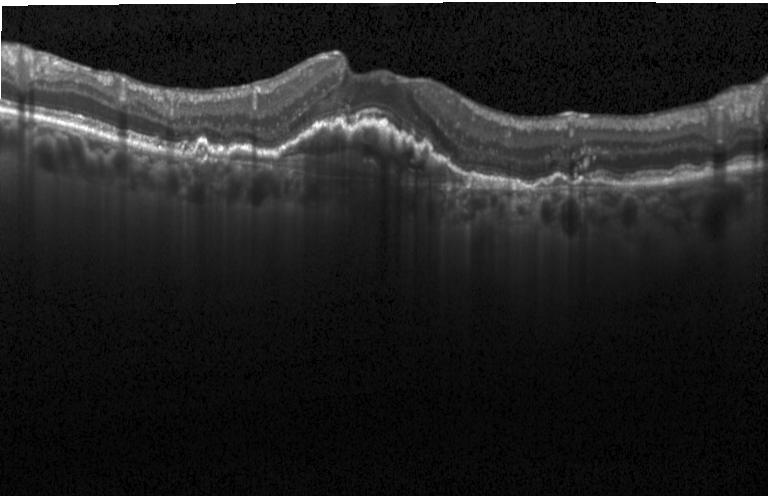 Optical coherence tomography scan
Macular OCT: a choroidal neovascular membrane.